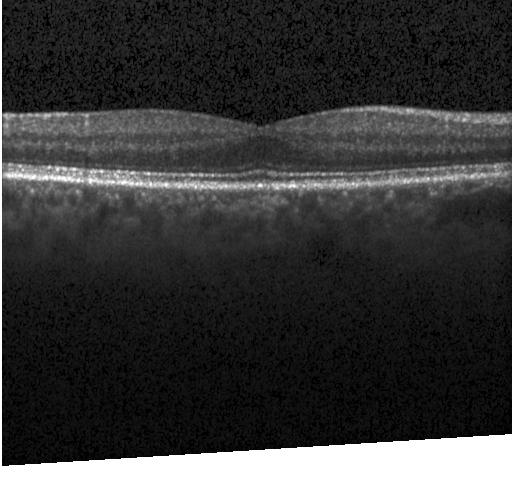

SD-OCT, OCT line scan — No choroidal neovascularization, no diabetic macular edema, and no drusen.